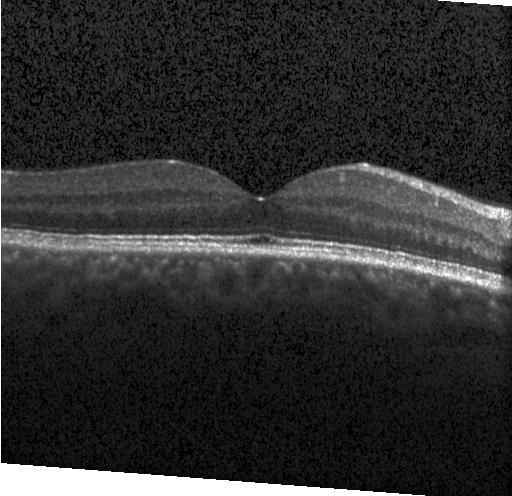

OCT B-scan · spectral-domain optical coherence tomography · through the macula · Heidelberg Spectralis.
Diagnosis: no choroidal neovascularization, diabetic macular edema, or drusen.